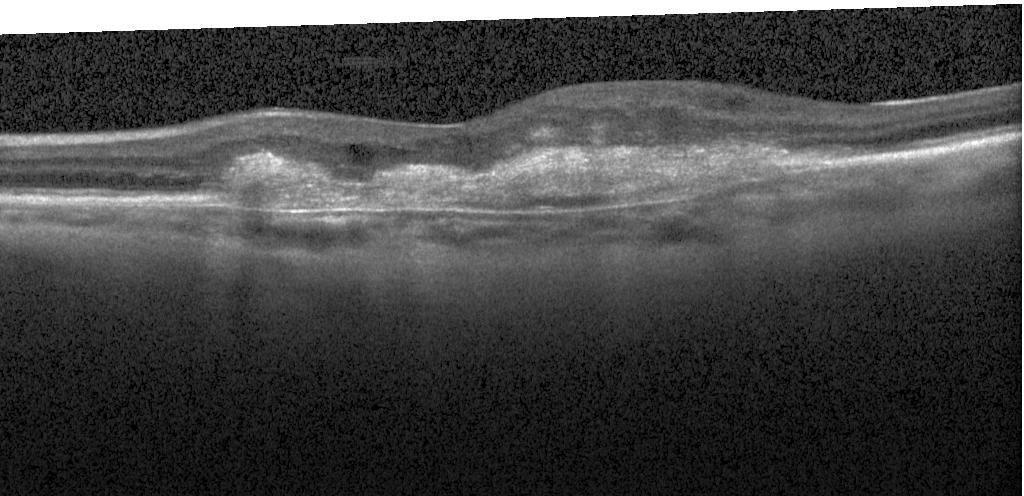
Assessment: a choroidal neovascular membrane.